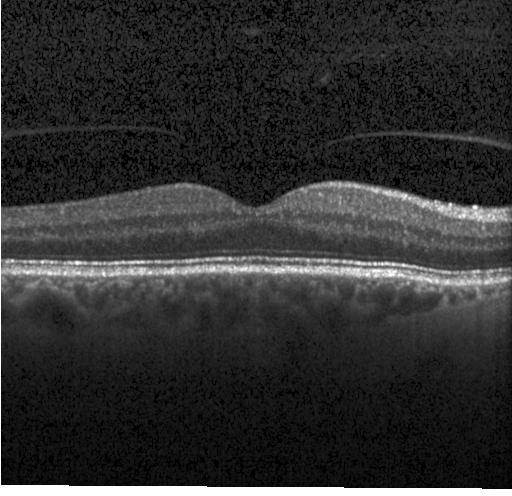 Assessment: neither choroidal neovascularization, diabetic macular edema, nor drusen.